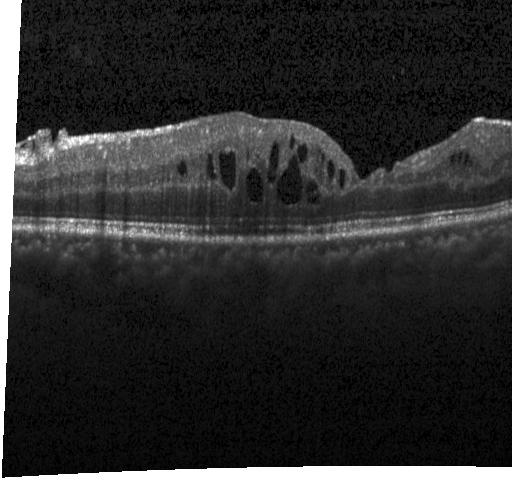 OCT finding: DME.